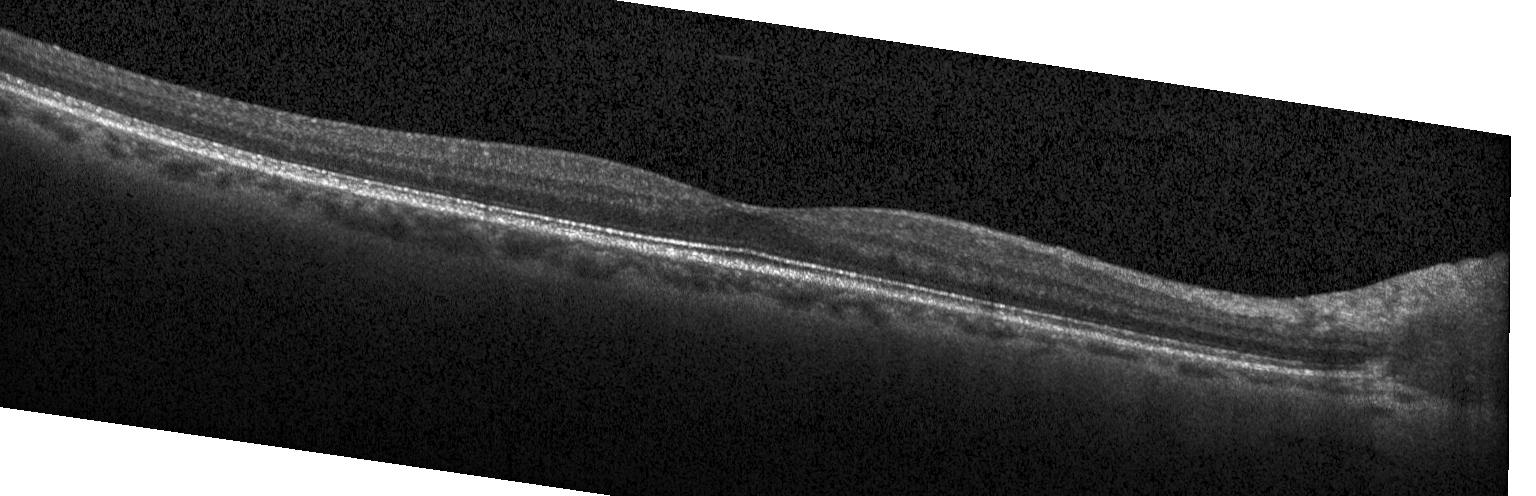

Retinal OCT cross-section.
Impression: no choroidal neovascularization, diabetic macular edema, or drusen.